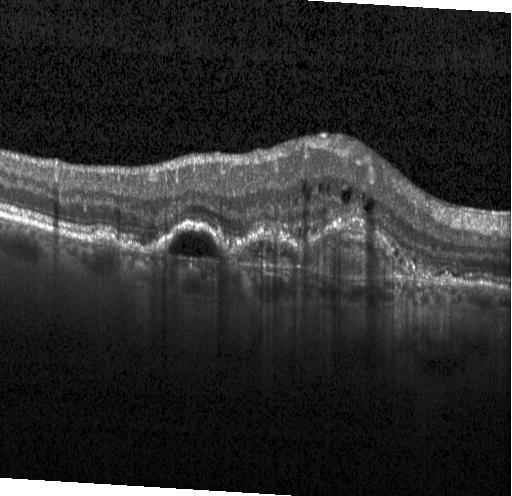
OCT B-scan, spectral-domain OCT, centered on the fovea — The scan shows a choroidal neovascular membrane.